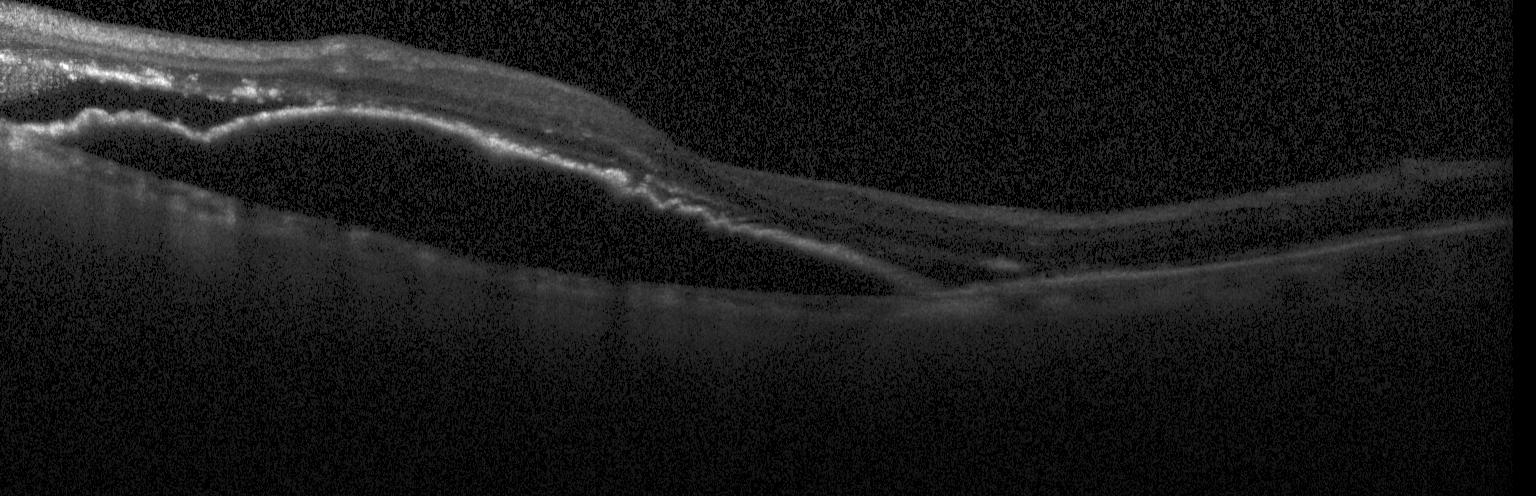
Heidelberg Spectralis; spectral-domain optical coherence tomography; fovea-centered; OCT B-scan — Dx: choroidal neovascularization (CNV).